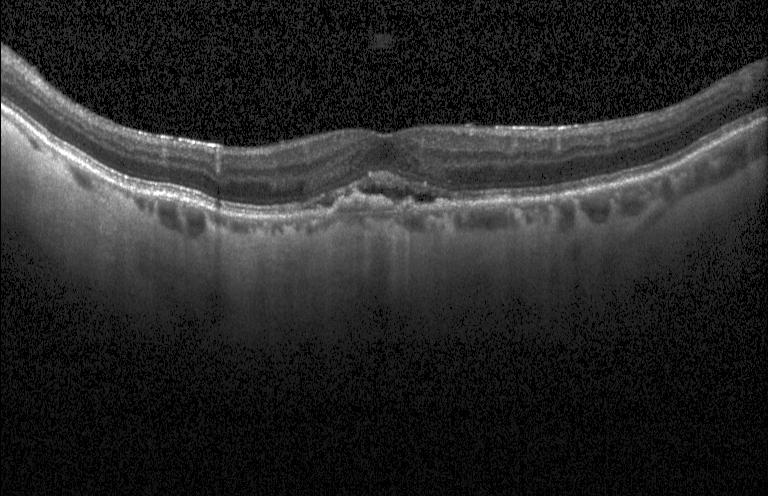 Diagnosis: a choroidal neovascular membrane.